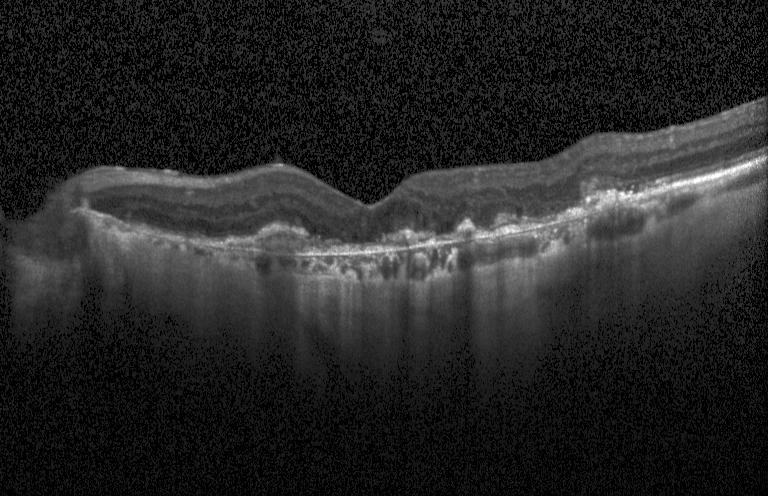

OCT B-scan.
This B-scan demonstrates choroidal neovascularization.